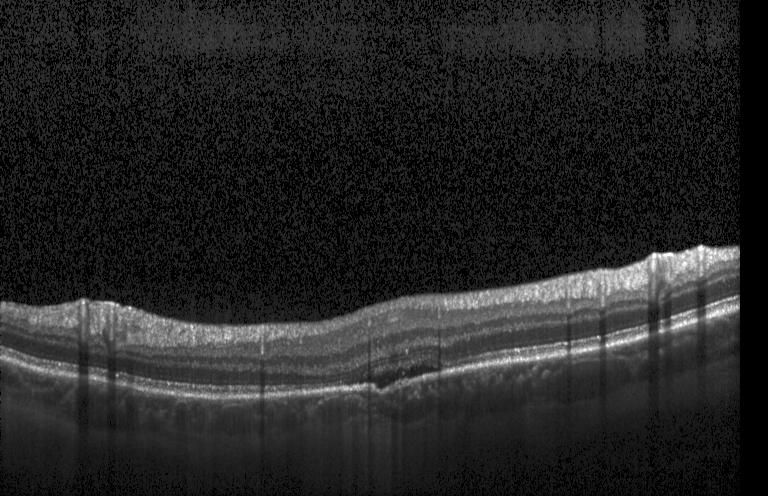

Assessment: choroidal neovascularization.